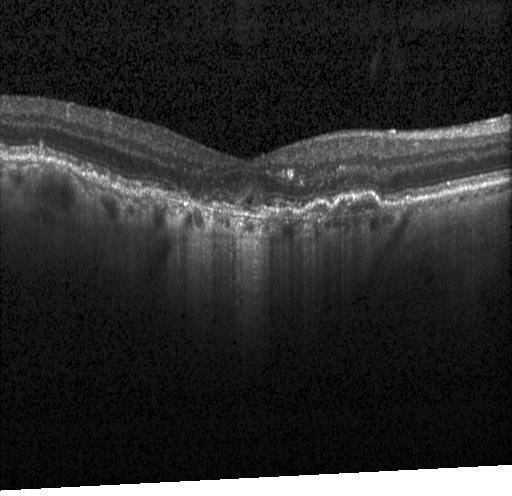

Macular OCT demonstrating a choroidal neovascular membrane.